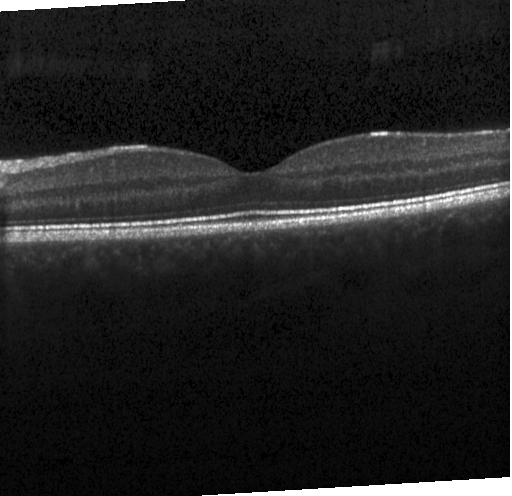

Spectral-domain optical coherence tomography · Heidelberg Spectralis · retinal OCT B-scan.
Dx: no choroidal neovascularization, diabetic macular edema, or drusen.